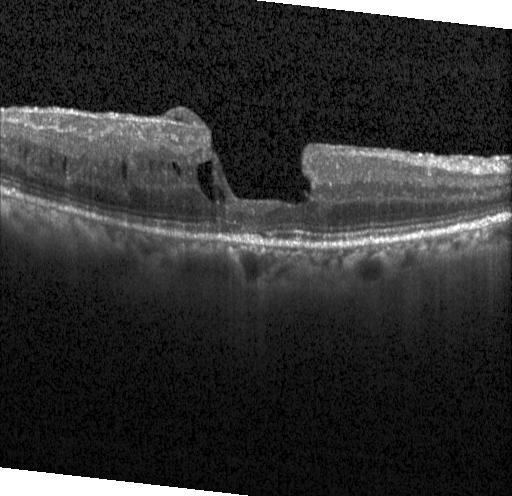 Optical coherence tomography B-scan. SD-OCT
Macular OCT: diabetic macular edema (DME).